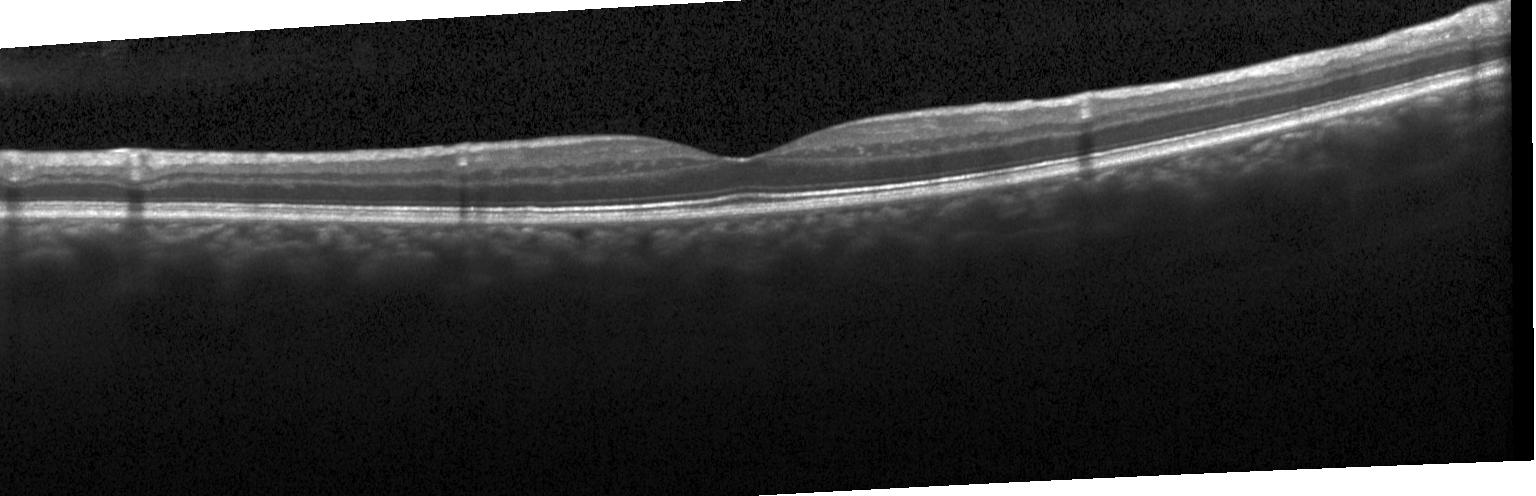

Acquired on a Heidelberg Spectralis · OCT B-scan. Assessment: no CNV, DME, or drusen.